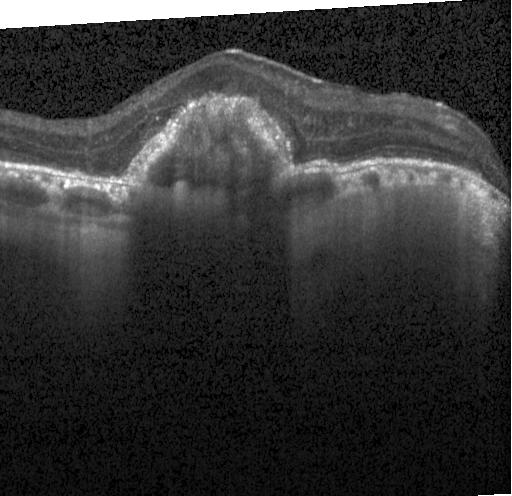 This B-scan demonstrates choroidal neovascularization.